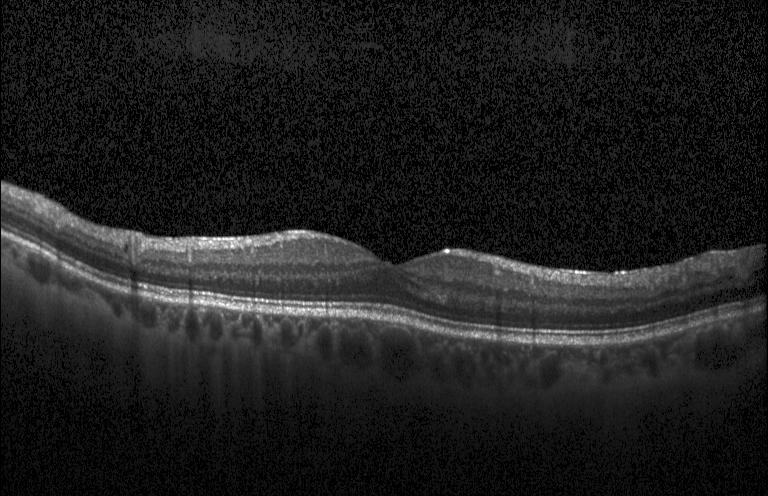 OCT finding: no choroidal neovascularization, diabetic macular edema, or drusen.